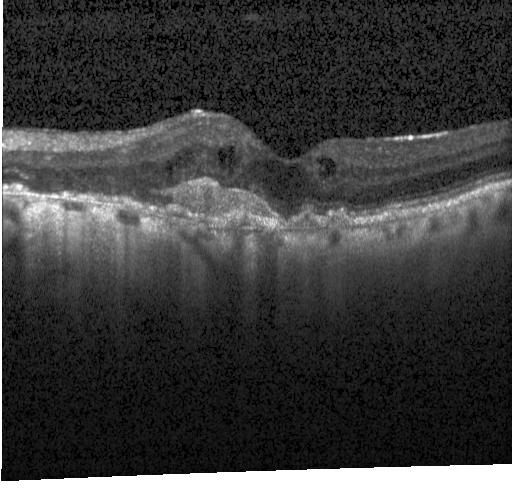
Acquired on a Heidelberg Spectralis; optical coherence tomography scan. Impression: a choroidal neovascular membrane.